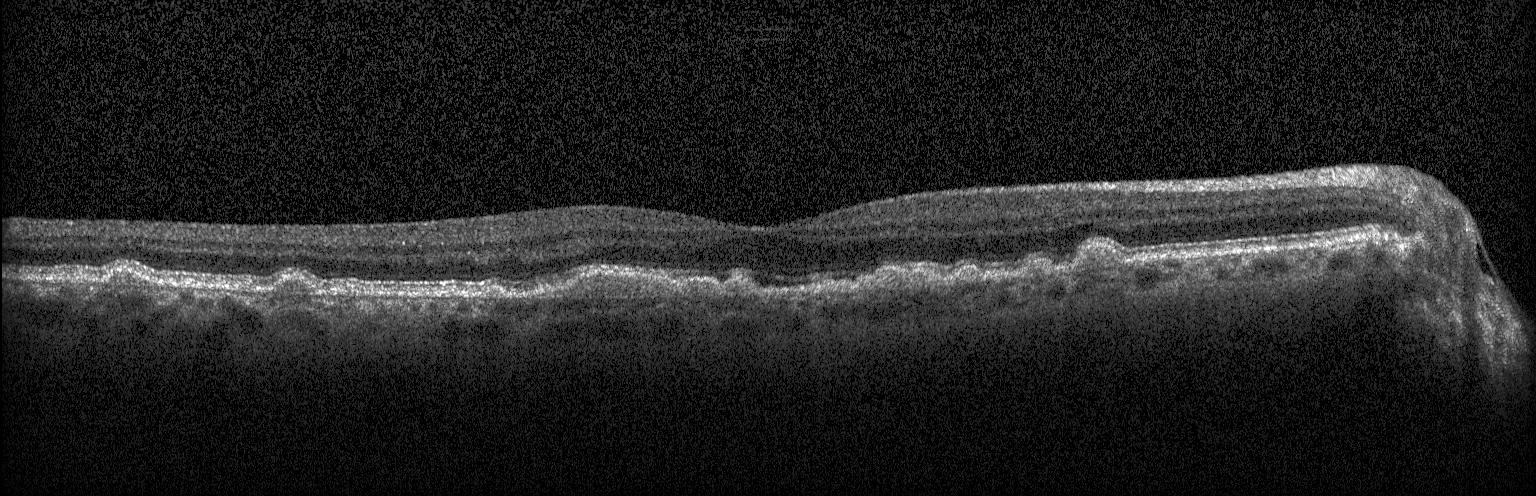
Spectral-domain OCT, macular scan, retinal OCT cross-section — The scan shows multiple drusen.